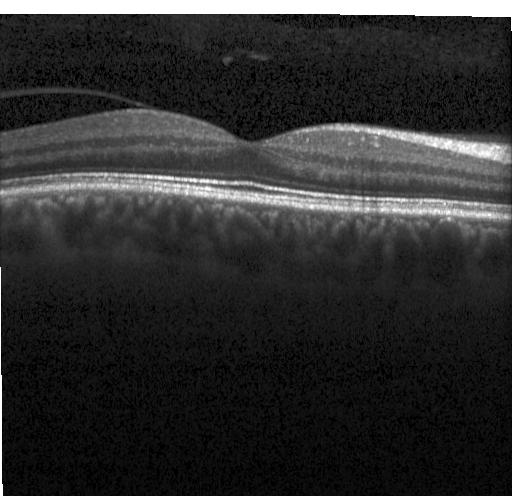

Spectral-domain OCT B-scan: no evidence of CNV, DME, or drusen.